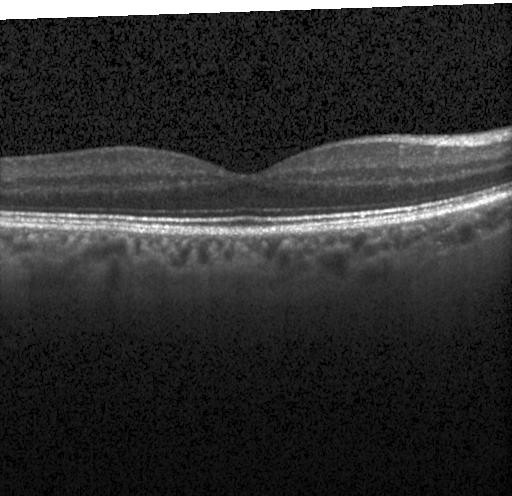

Diagnosis: no evidence of choroidal neovascularization, diabetic macular edema, or drusen.